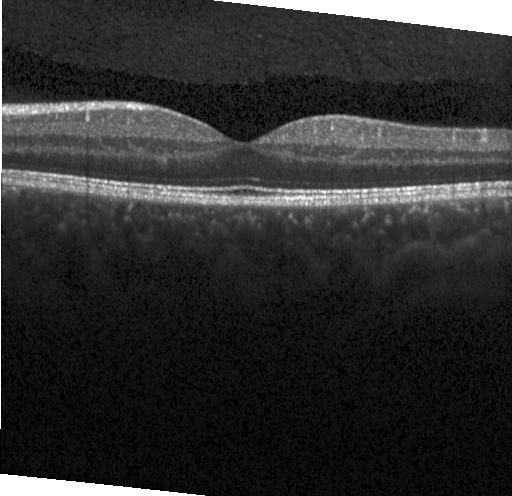

Instrument: Heidelberg Spectralis · spectral-domain optical coherence tomography · OCT B-scan · macular scan
Finding: no evidence of CNV, DME, or drusen.